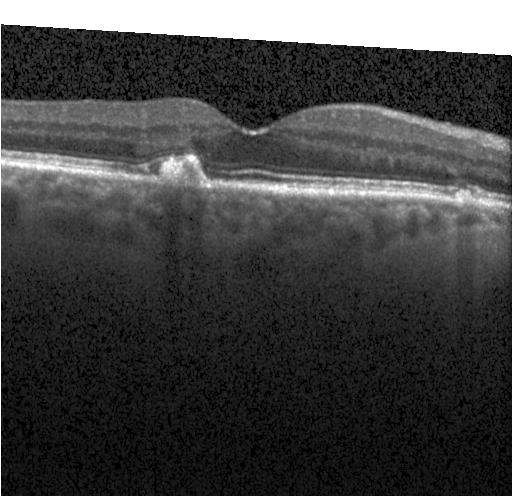 OCT B-scan
This B-scan demonstrates a choroidal neovascular membrane.